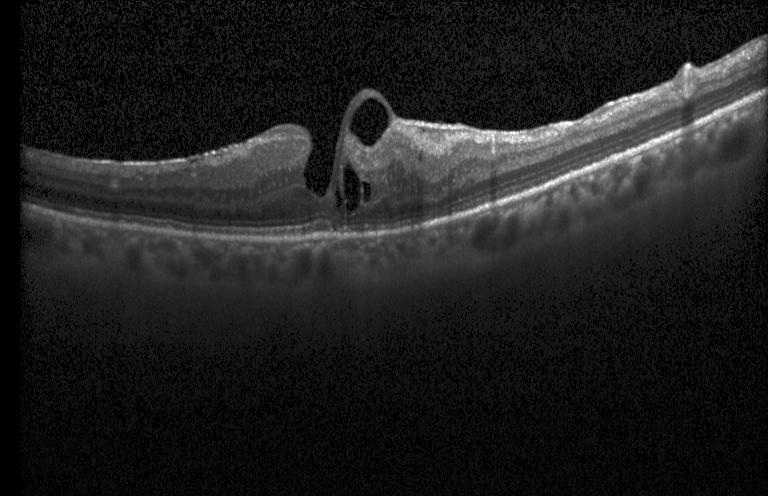

Optical coherence tomography B-scan
Impression: diabetic macular edema (DME).